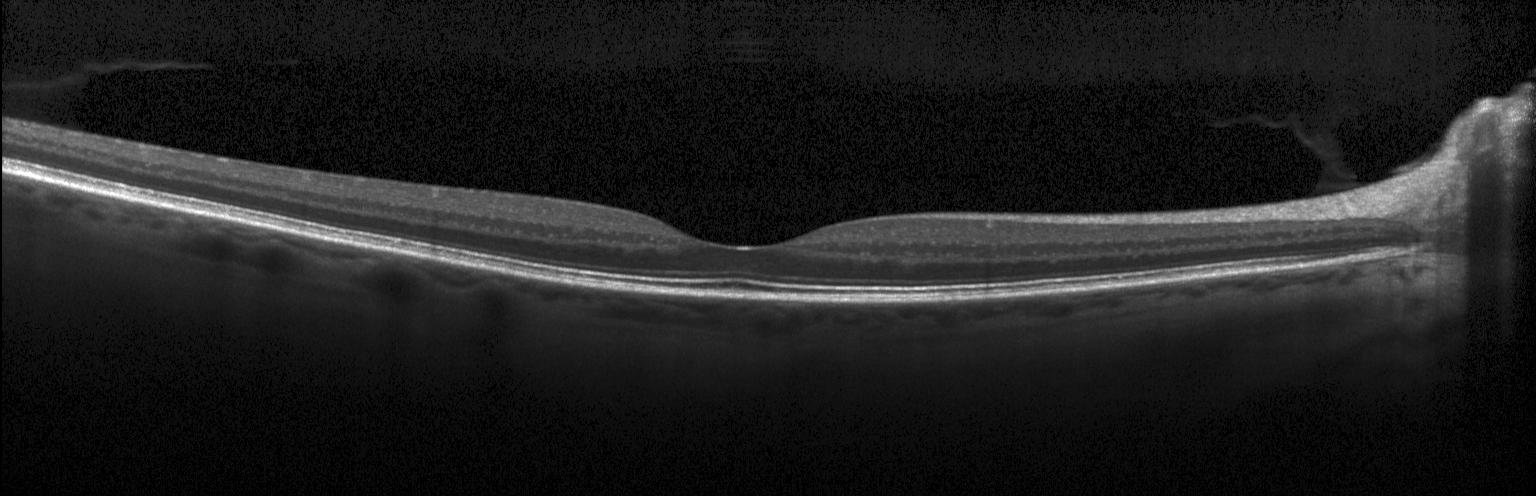 Impression: no choroidal neovascularization, no diabetic macular edema, and no drusen.